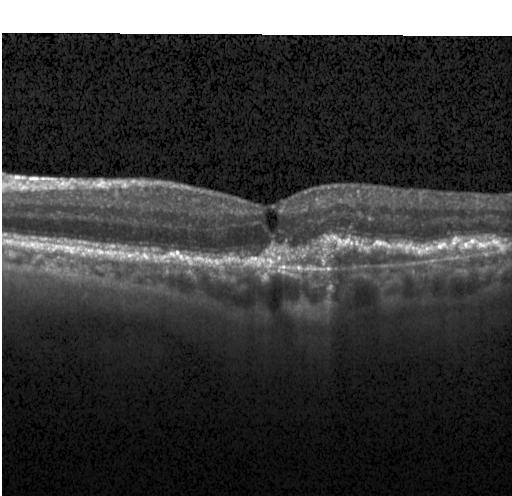 Retinal OCT B-scan · spectral-domain OCT · centered on the fovea — Dx: choroidal neovascularization.